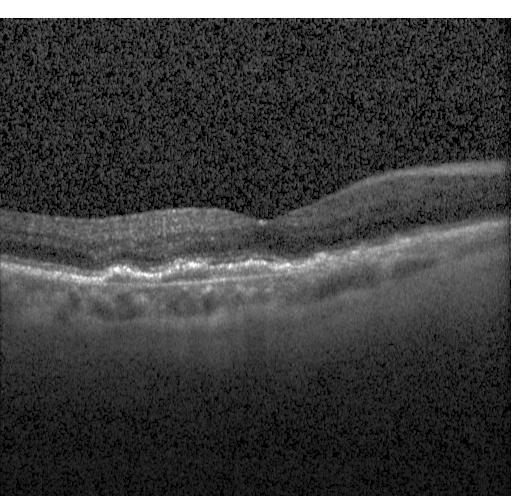

OCT B-scan · Heidelberg Spectralis OCT system.
Finding: a choroidal neovascular membrane.